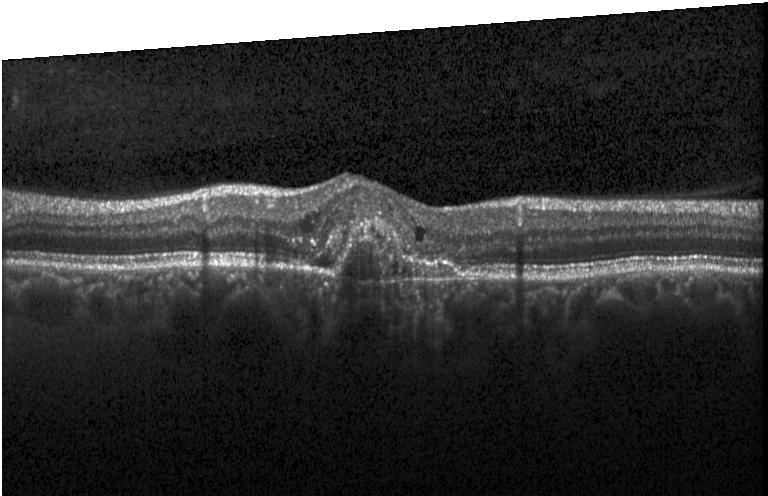
Horizontal scan through the fovea · acquired on a Heidelberg Spectralis · OCT line scan.
Impression: a choroidal neovascular membrane.